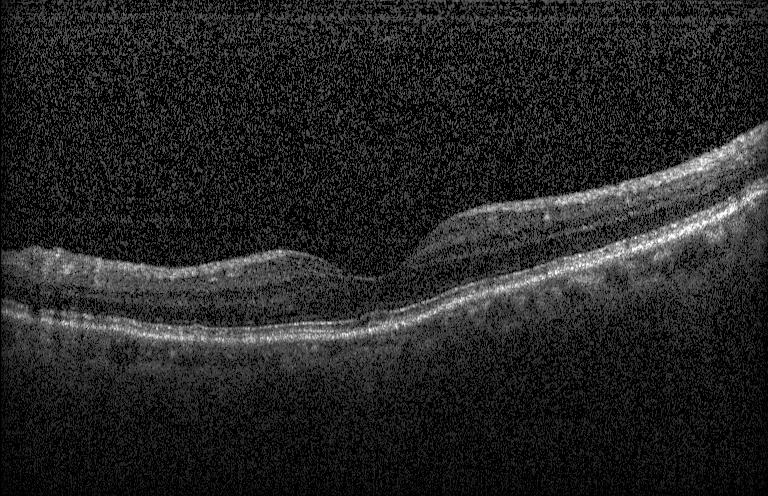

Retinal OCT cross-section; spectral-domain optical coherence tomography. Finding: no evidence of choroidal neovascularization, diabetic macular edema, or drusen.